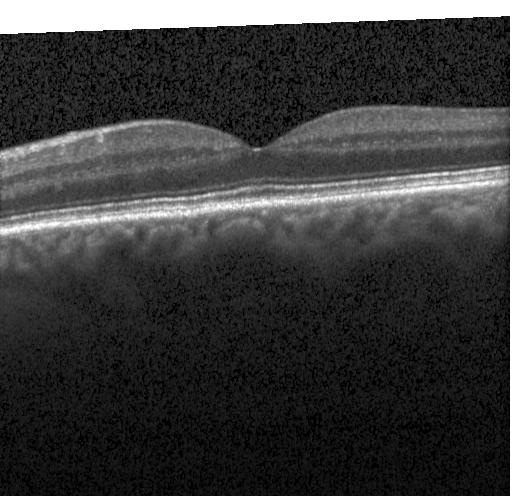
OCT B-scan · macular scan.
Finding: no evidence of CNV, DME, or drusen.